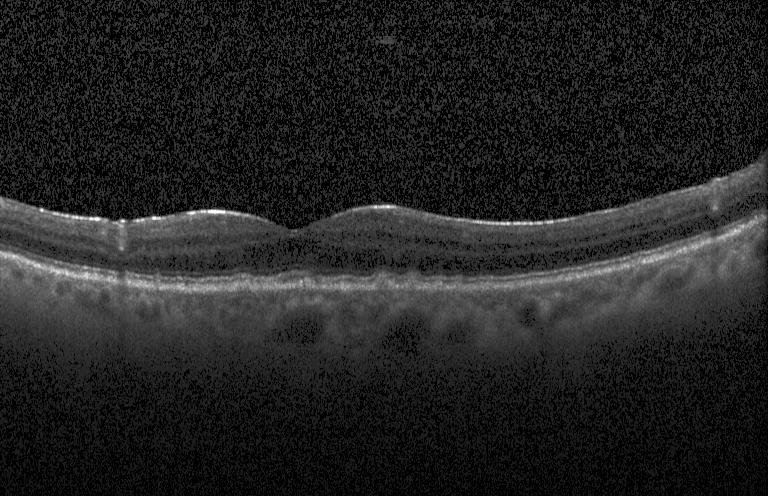
Macular OCT: multiple drusen.